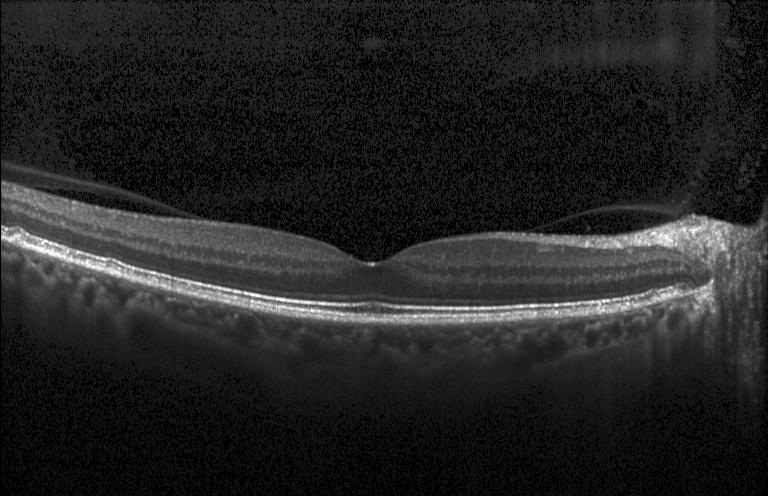
Optical coherence tomography B-scan; spectral-domain OCT; acquired on a Heidelberg Spectralis; macular scan. Macular OCT: no choroidal neovascularization, no diabetic macular edema, and no drusen.